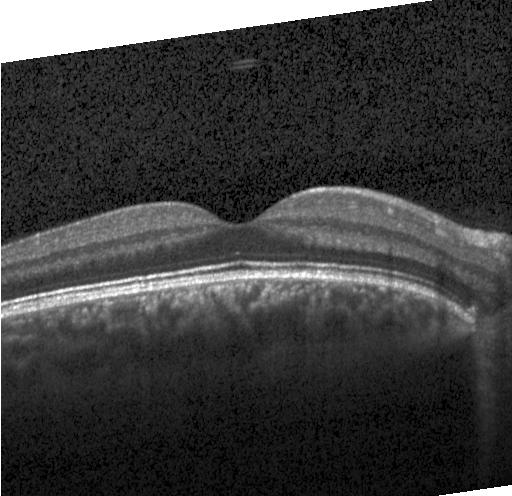
Spectral-domain optical coherence tomography · retinal OCT B-scan · centered on the fovea · instrument: Heidelberg Spectralis. The scan shows neither choroidal neovascularization, diabetic macular edema, nor drusen.